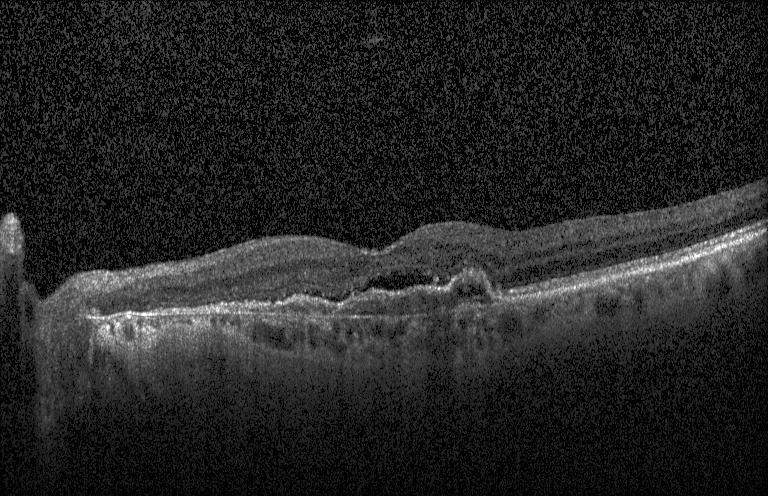

Finding: a choroidal neovascular membrane.